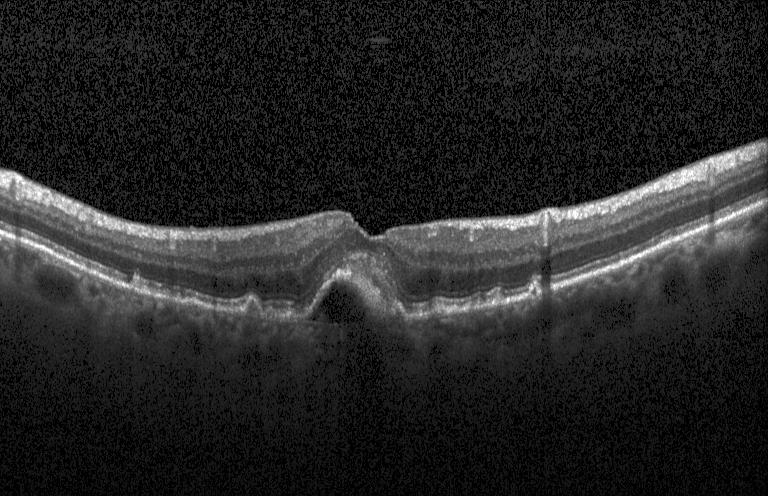

Spectral-domain optical coherence tomography · optical coherence tomography B-scan · fovea-centered · instrument: Heidelberg Spectralis.
Diagnosis: CNV.